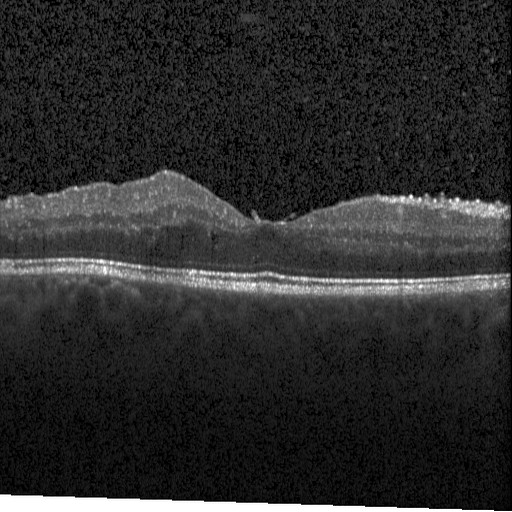 Impression: DME.